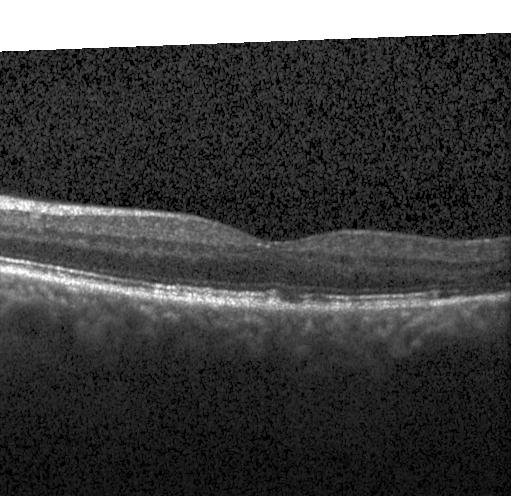
Centered on the fovea. Instrument: Heidelberg Spectralis. Retinal OCT B-scan.
Impression: sub-RPE drusenoid deposits.